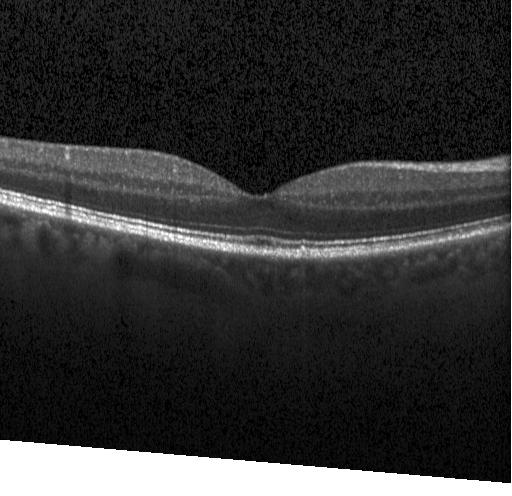
Centered on the fovea. Spectral-domain OCT. OCT B-scan — This B-scan demonstrates no evidence of choroidal neovascularization, diabetic macular edema, or drusen.